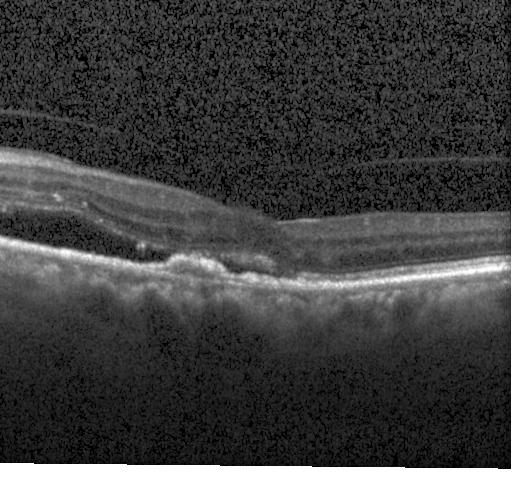 SD-OCT · fovea-centered · OCT B-scan
Impression: a choroidal neovascular membrane.